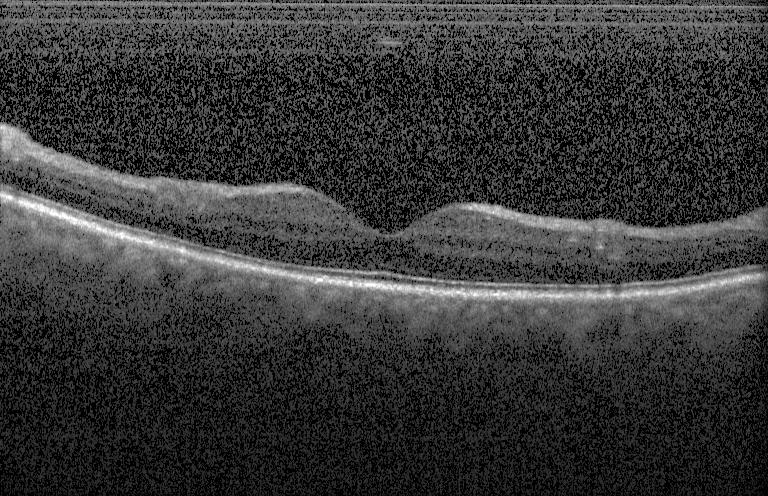 Diagnosis: no evidence of choroidal neovascularization, diabetic macular edema, or drusen.